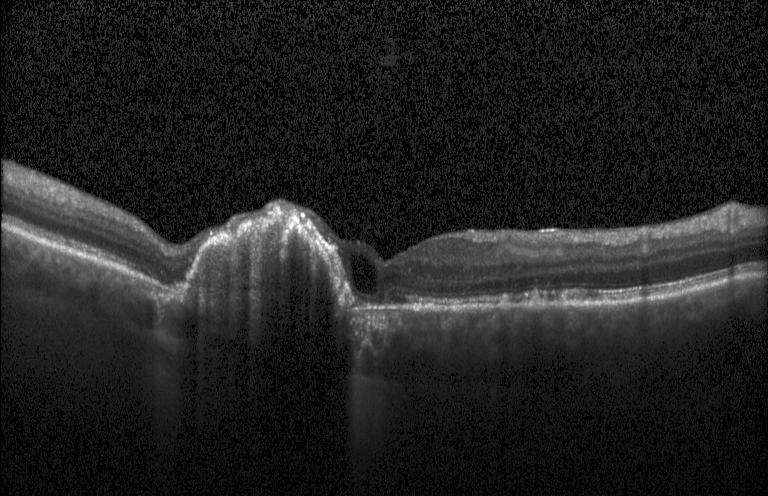 Retinal OCT B-scan.
CNV.